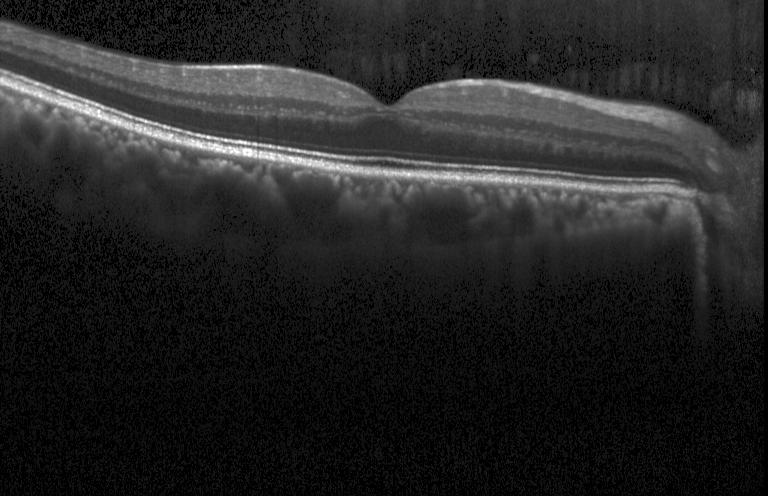
Optical coherence tomography scan, spectral-domain optical coherence tomography. No choroidal neovascularization, no diabetic macular edema, and no drusen.